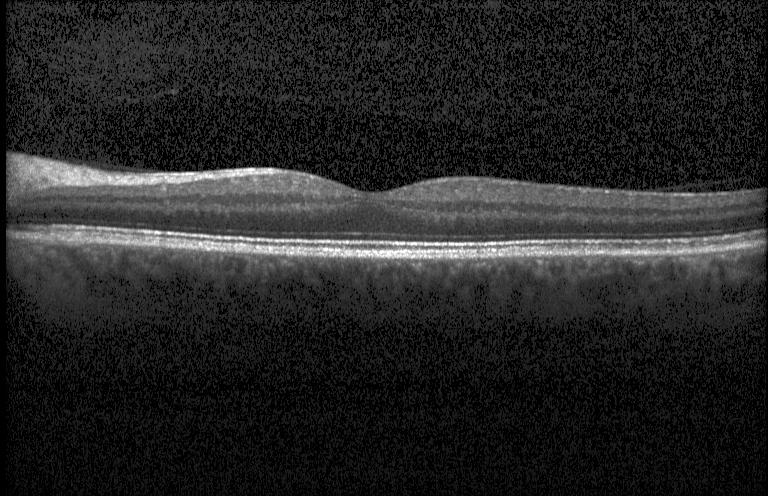

Finding: no evidence of choroidal neovascularization, diabetic macular edema, or drusen.